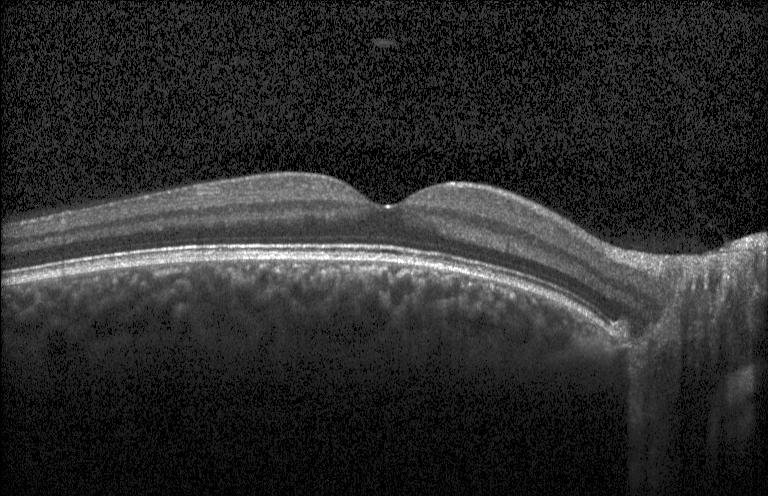 Optical coherence tomography B-scan
Dx: no choroidal neovascularization, no diabetic macular edema, and no drusen.